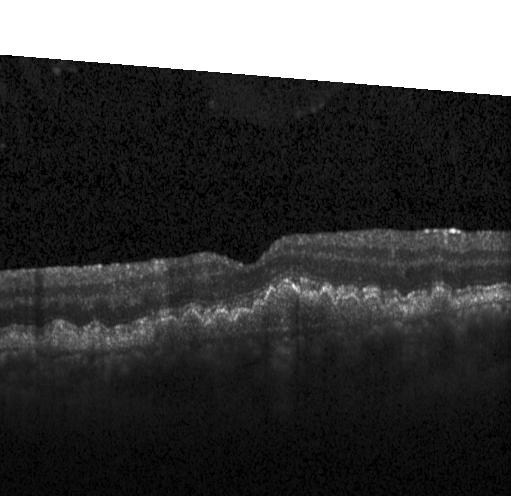

Impression: a choroidal neovascular membrane.